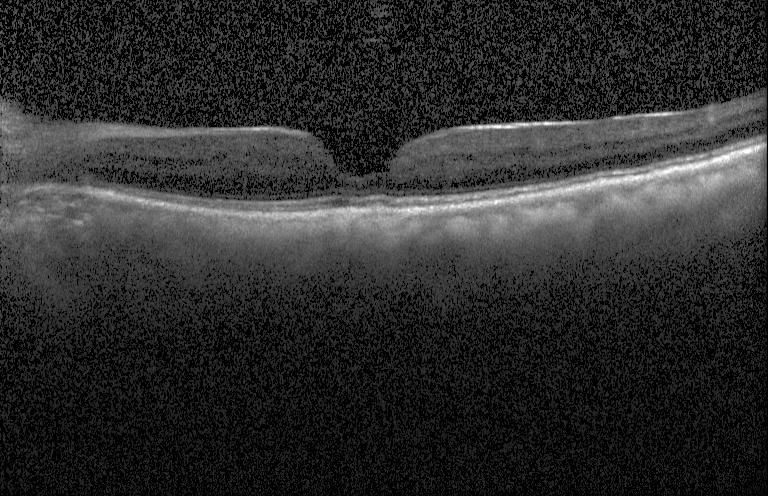

Optical coherence tomography B-scan; through the macula
Finding: neither choroidal neovascularization, diabetic macular edema, nor drusen.